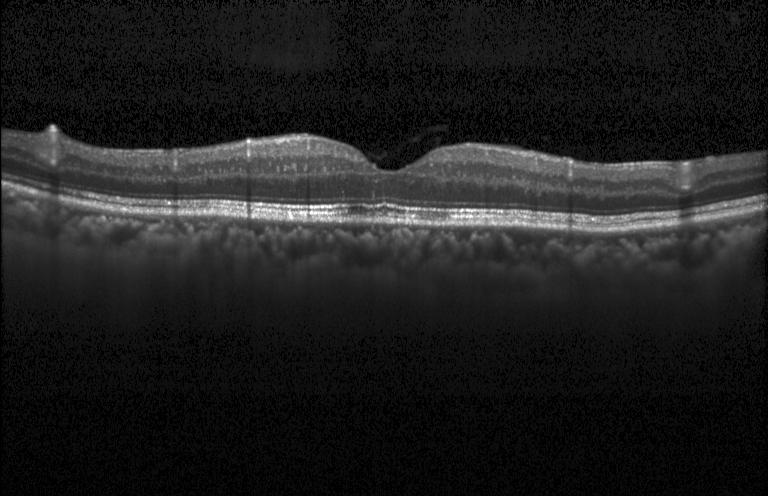

Fovea-centered · spectral-domain OCT · retinal OCT B-scan · Heidelberg Spectralis OCT system.
OCT finding: no choroidal neovascularization, no diabetic macular edema, and no drusen.